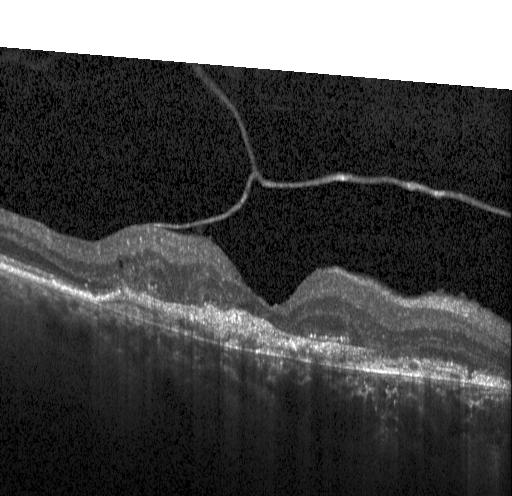 The scan shows a choroidal neovascular membrane.